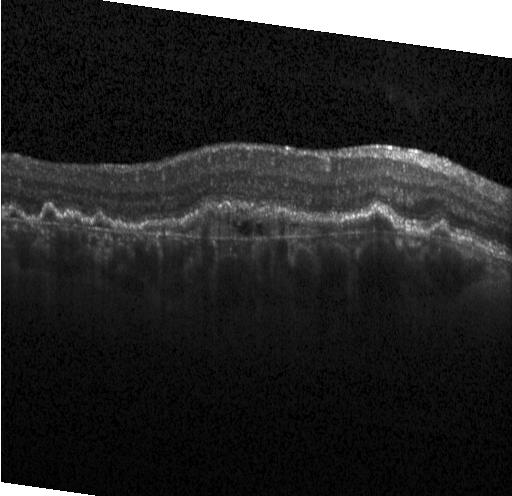

A choroidal neovascular membrane.